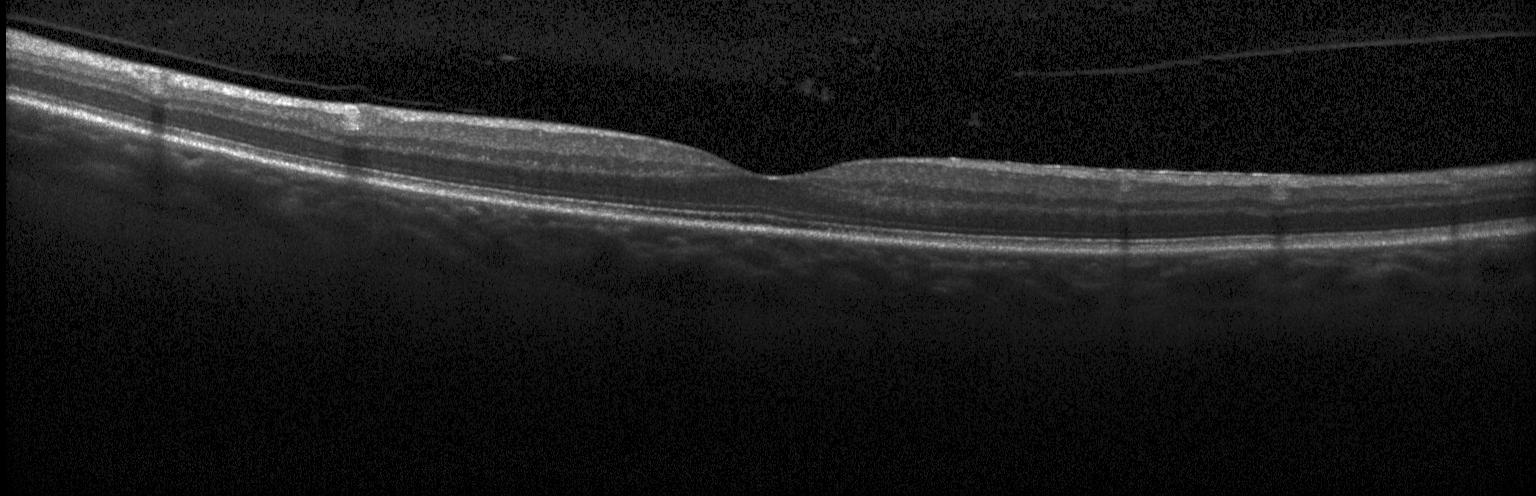 OCT scan showing neither choroidal neovascularization, diabetic macular edema, nor drusen.